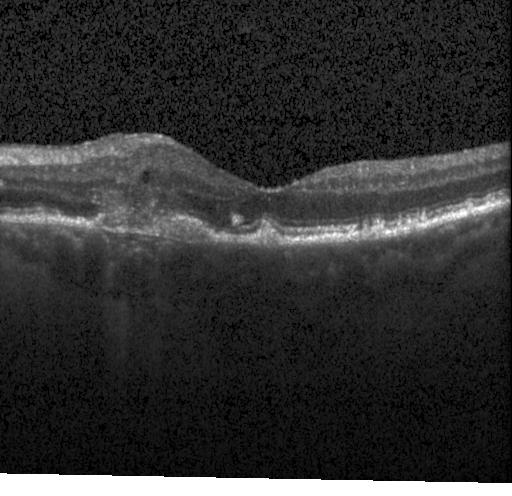

SD-OCT; Heidelberg Spectralis OCT system; macular scan; OCT B-scan.
Finding: choroidal neovascularization (CNV).